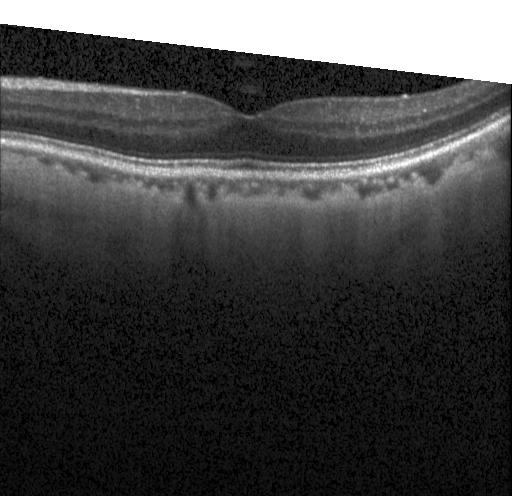
Macular scan; OCT line scan
Diagnosis: no choroidal neovascularization, no diabetic macular edema, and no drusen.